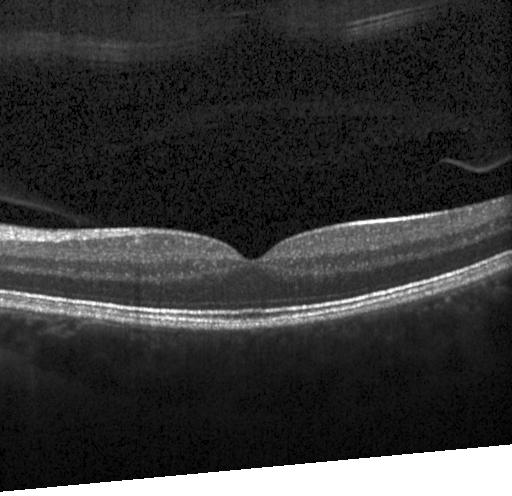
Optical coherence tomography B-scan
Diagnosis: no CNV, no DME, and no drusen.